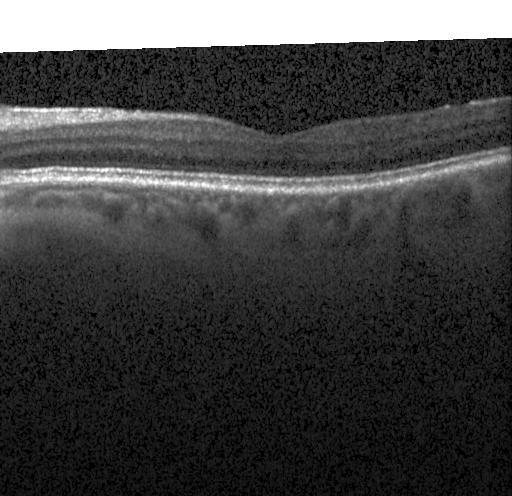
Macular OCT: no choroidal neovascularization, no diabetic macular edema, and no drusen.